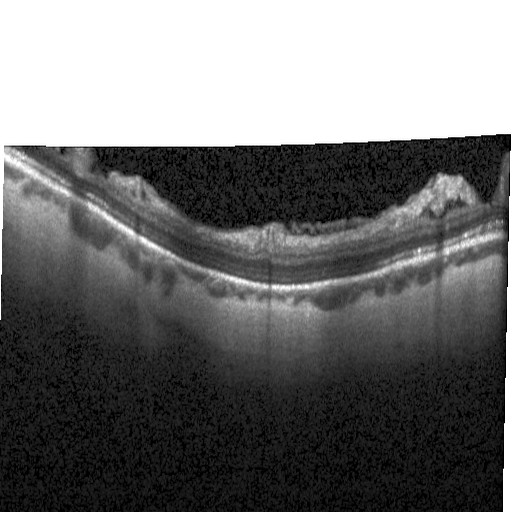
Instrument: Heidelberg Spectralis · retinal OCT cross-section — Finding: diabetic macular edema (DME).